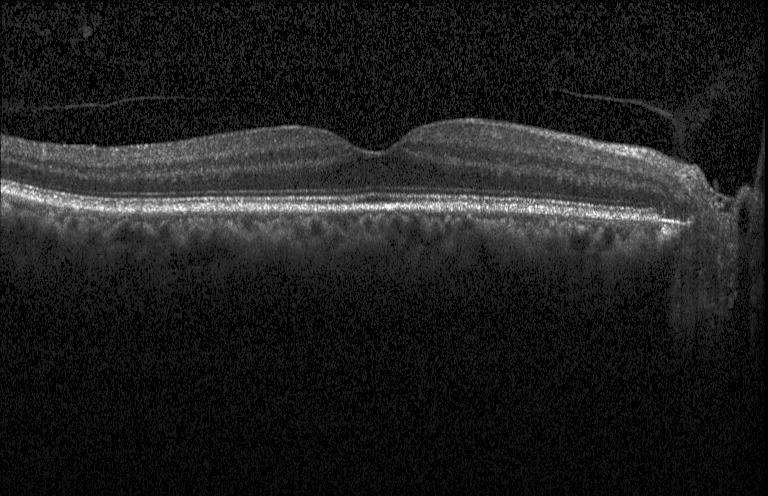
Diagnosis: no evidence of choroidal neovascularization, diabetic macular edema, or drusen.